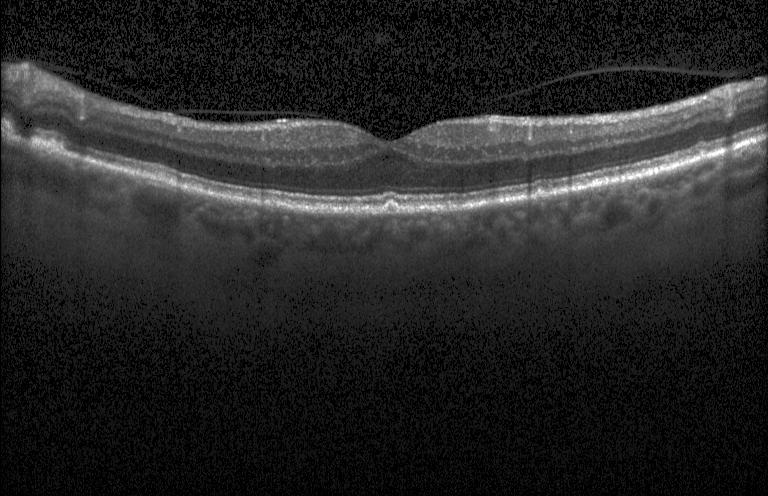 Spectral-domain optical coherence tomography. Macular scan. Retinal OCT B-scan.
The scan shows multiple drusen.